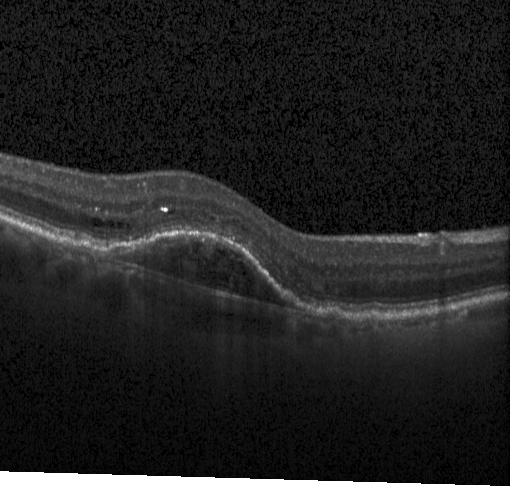

CNV.